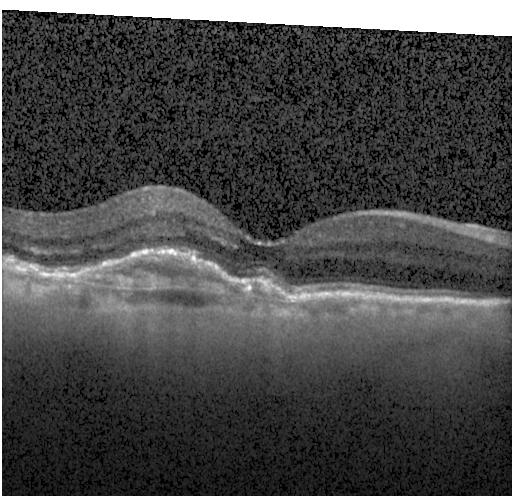

Retinal OCT B-scan, horizontal scan through the fovea
OCT finding: a choroidal neovascular membrane.